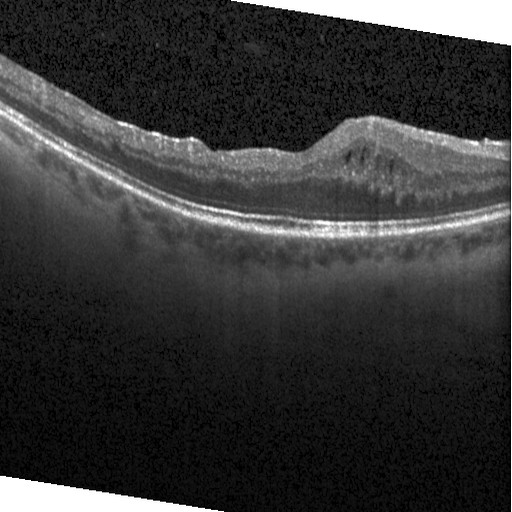

OCT line scan; SD-OCT; fovea-centered; acquired on a Heidelberg Spectralis.
Diabetic macular edema (DME).